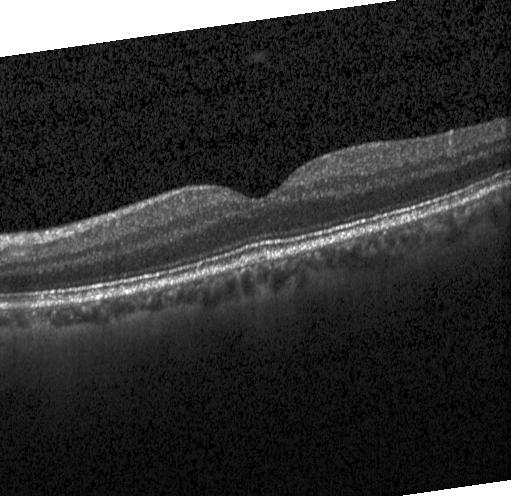 Retinal OCT cross-section.
Diagnosis: neither choroidal neovascularization, diabetic macular edema, nor drusen.